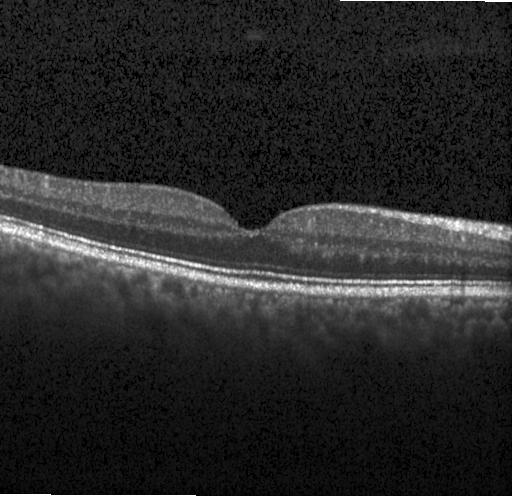
OCT finding: no choroidal neovascularization, diabetic macular edema, or drusen.